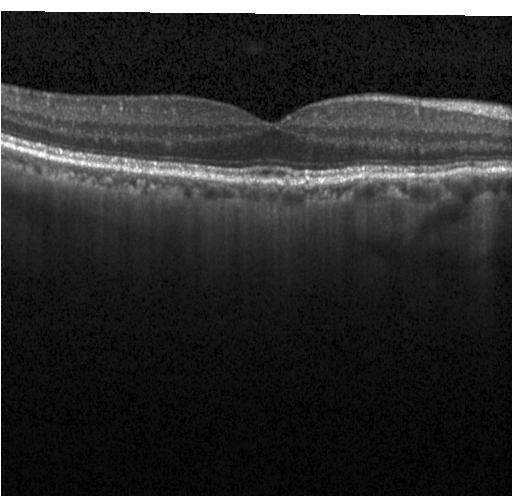
Centered on the fovea · spectral-domain OCT · Heidelberg Spectralis · optical coherence tomography scan — Sub-RPE drusenoid deposits.